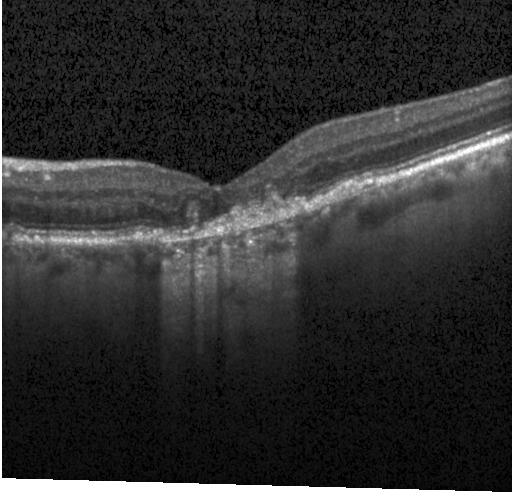

Retinal OCT cross-section showing choroidal neovascularization (CNV).